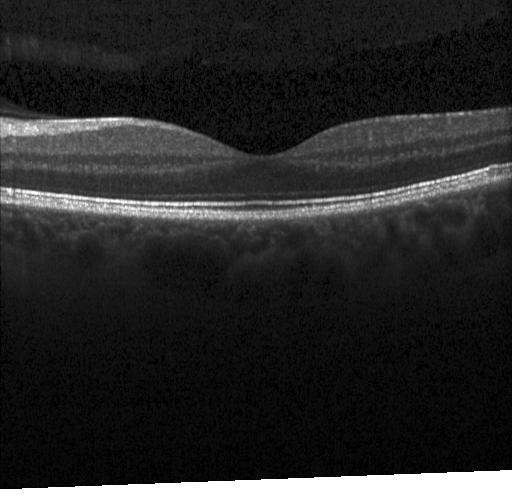
Diagnosis: no evidence of choroidal neovascularization, diabetic macular edema, or drusen.